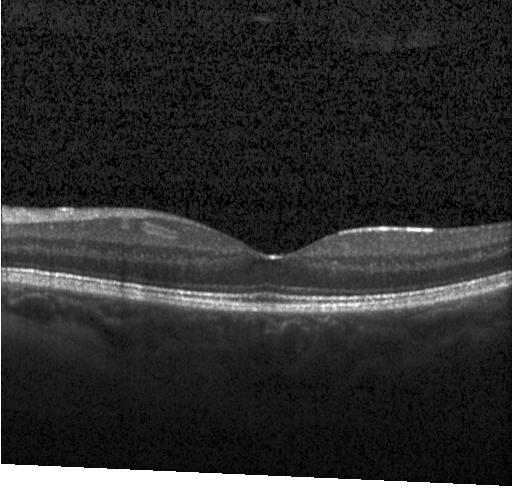
OCT B-scan. Spectral-domain optical coherence tomography. Fovea-centered. The scan shows no CNV, no DME, and no drusen.